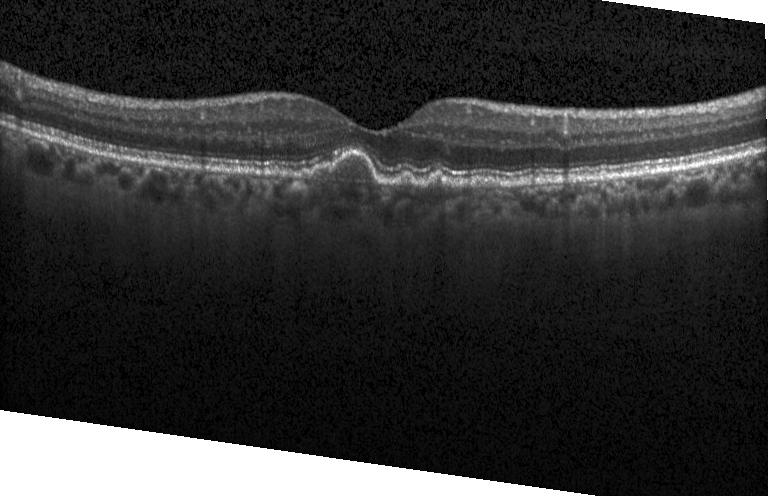
Retinal OCT B-scan. Assessment: multiple drusen.